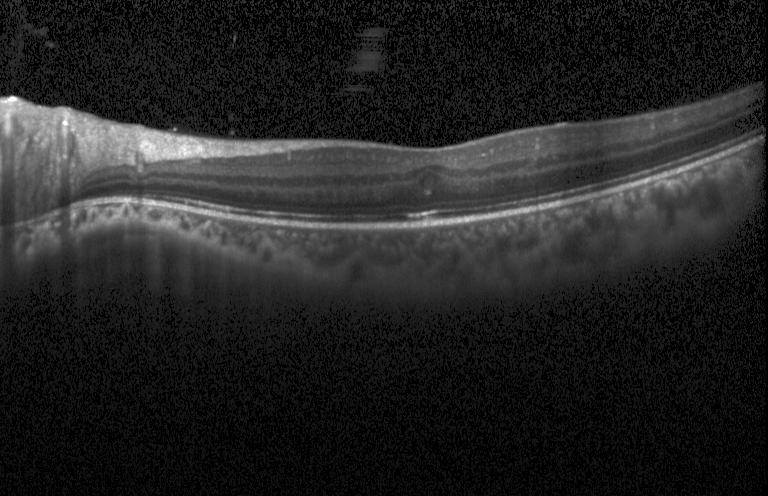 Finding: no choroidal neovascularization, no diabetic macular edema, and no drusen.